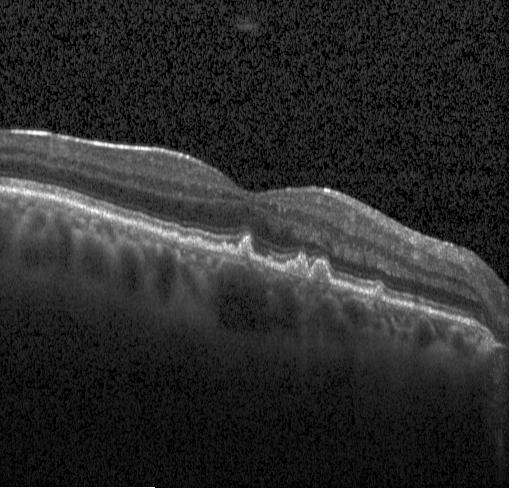
Through the macula. OCT line scan. Heidelberg Spectralis
Diagnosis: sub-RPE drusenoid deposits.